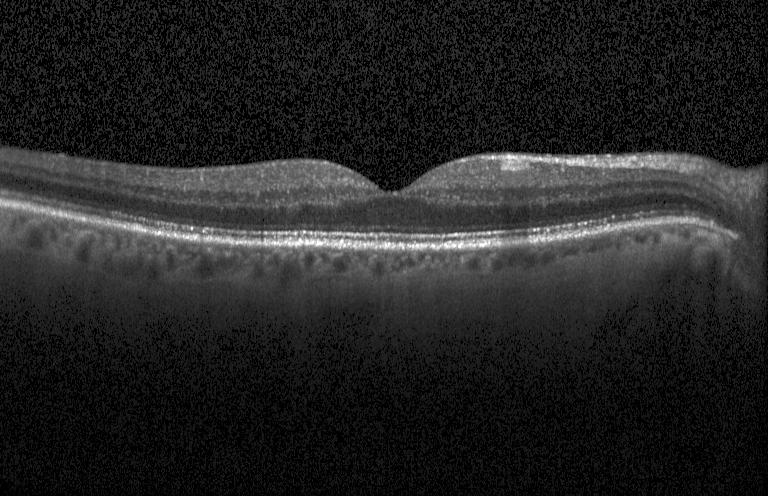 Diagnosis: no CNV, no DME, and no drusen.